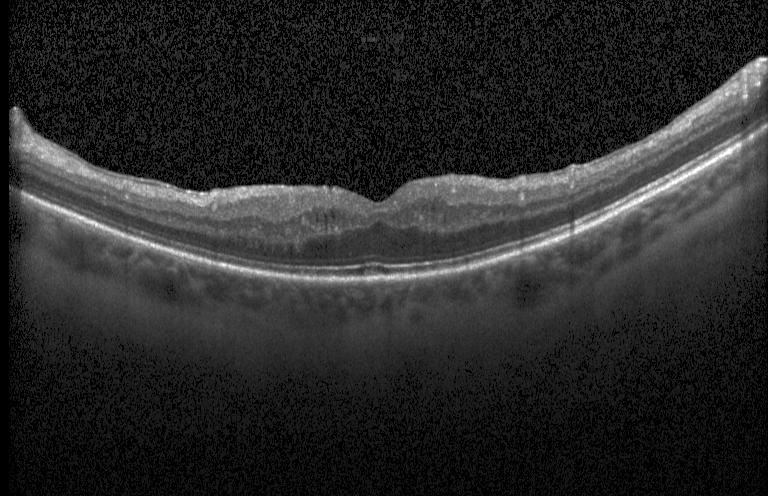 OCT line scan; Heidelberg Spectralis OCT system. Impression: diabetic macular edema (DME).